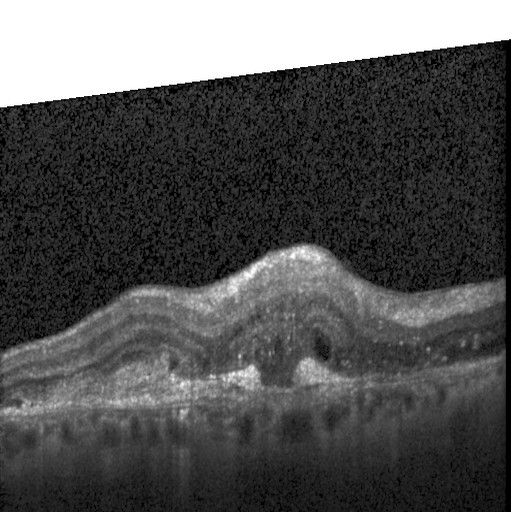 Diabetic macular edema (DME).